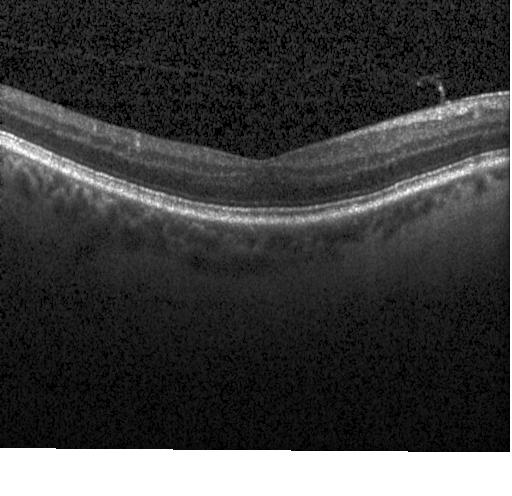
Neither CNV, DME, nor drusen.